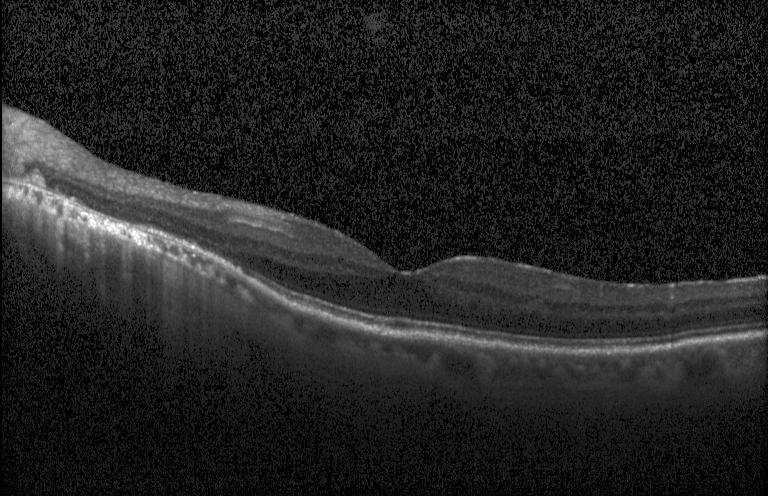
Centered on the fovea · optical coherence tomography scan. Finding: neither choroidal neovascularization, diabetic macular edema, nor drusen.